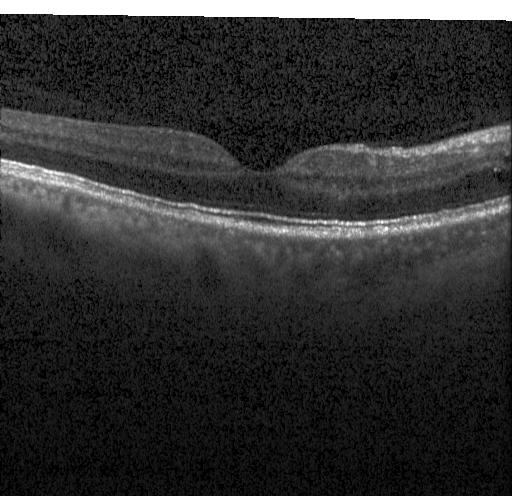 Impression: no evidence of choroidal neovascularization, diabetic macular edema, or drusen.